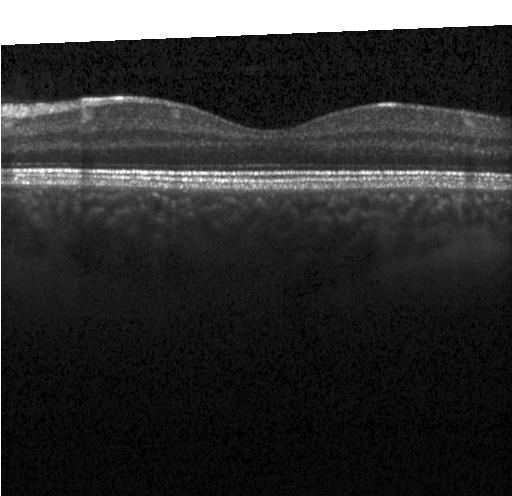 Assessment: neither choroidal neovascularization, diabetic macular edema, nor drusen.